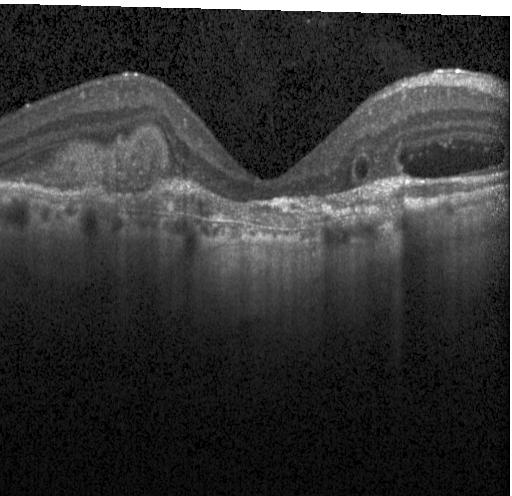
Centered on the fovea, OCT B-scan, Heidelberg Spectralis, SD-OCT. Assessment: a choroidal neovascular membrane.